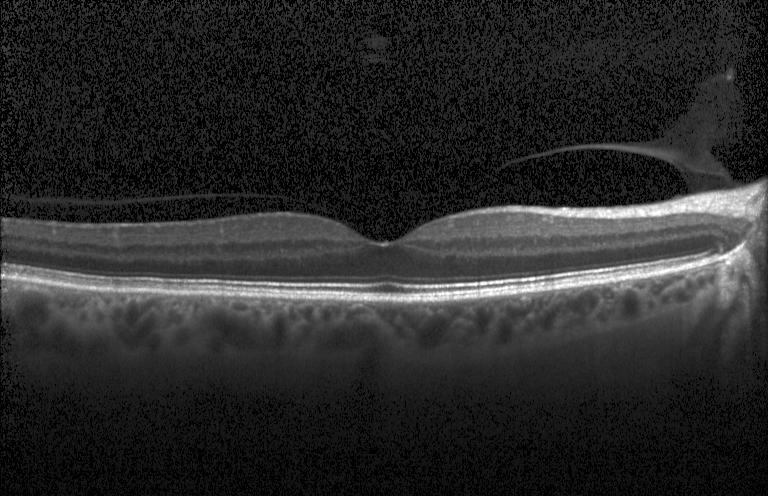
Diagnosis: neither choroidal neovascularization, diabetic macular edema, nor drusen.